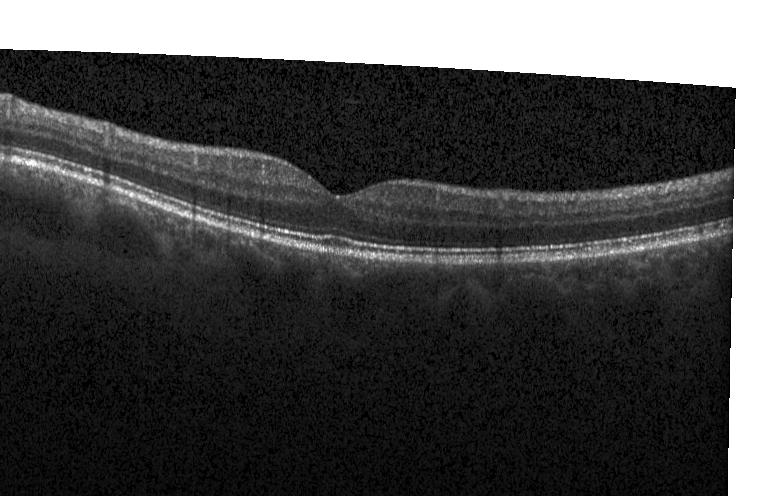

OCT line scan — Diagnosis: neither CNV, DME, nor drusen.